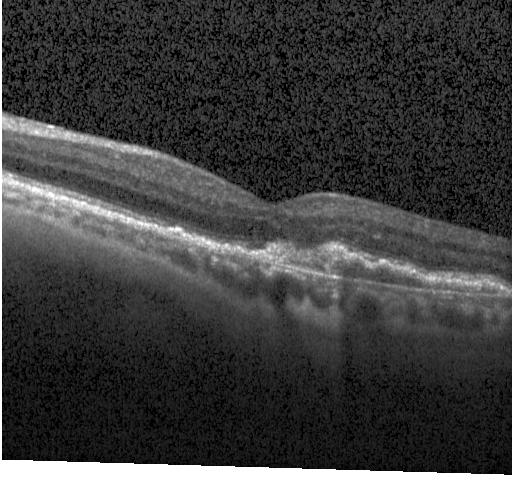
Impression: a choroidal neovascular membrane.